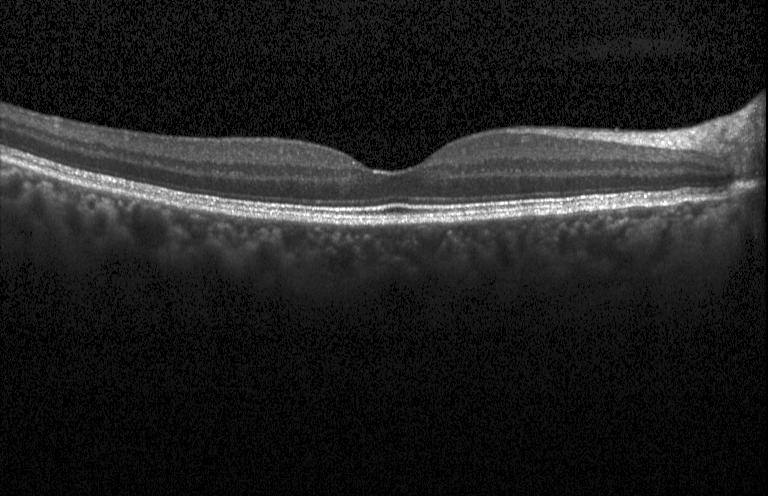

Macular OCT: neither choroidal neovascularization, diabetic macular edema, nor drusen.